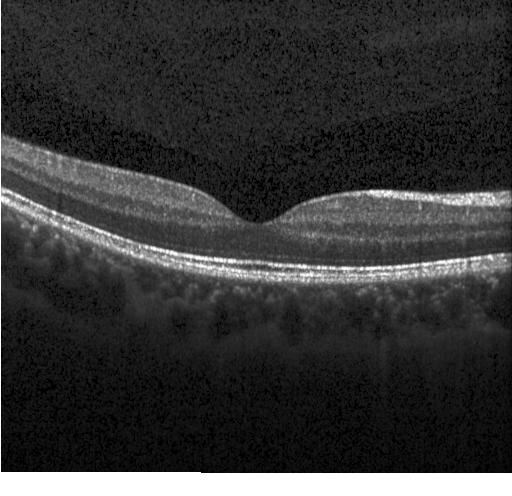 OCT finding: no choroidal neovascularization, no diabetic macular edema, and no drusen.